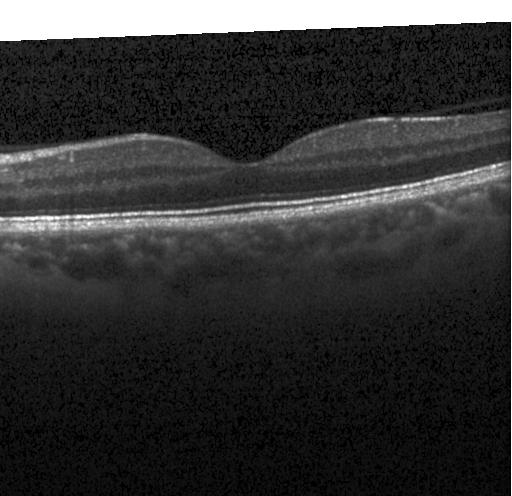 Optical coherence tomography scan, spectral-domain OCT, centered on the fovea, instrument: Heidelberg Spectralis. Finding: no CNV, no DME, and no drusen.